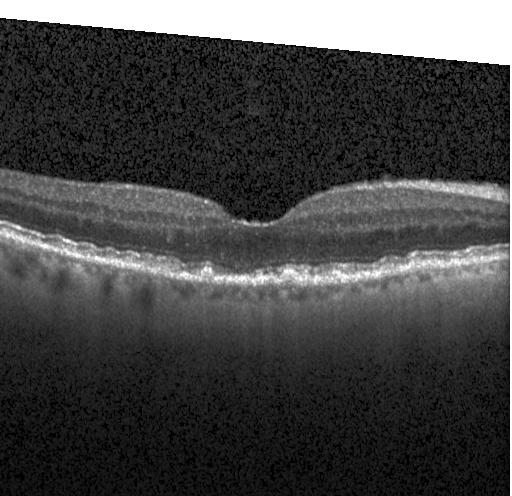
OCT B-scan showing drusen.